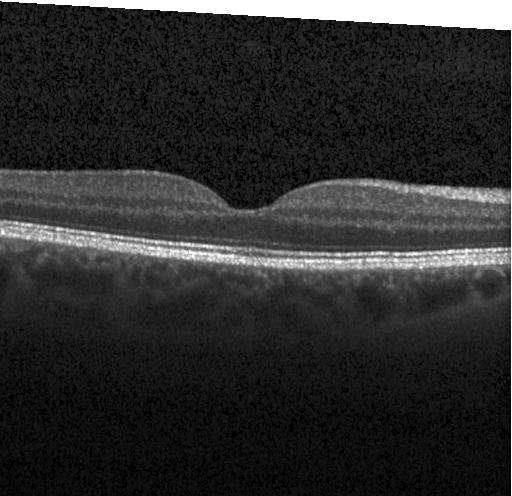
SD-OCT · acquired on a Heidelberg Spectralis · optical coherence tomography scan — Diagnosis: no CNV, DME, or drusen.